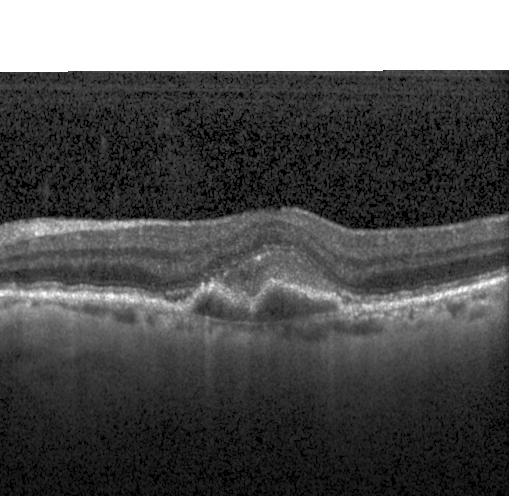

The scan shows CNV.